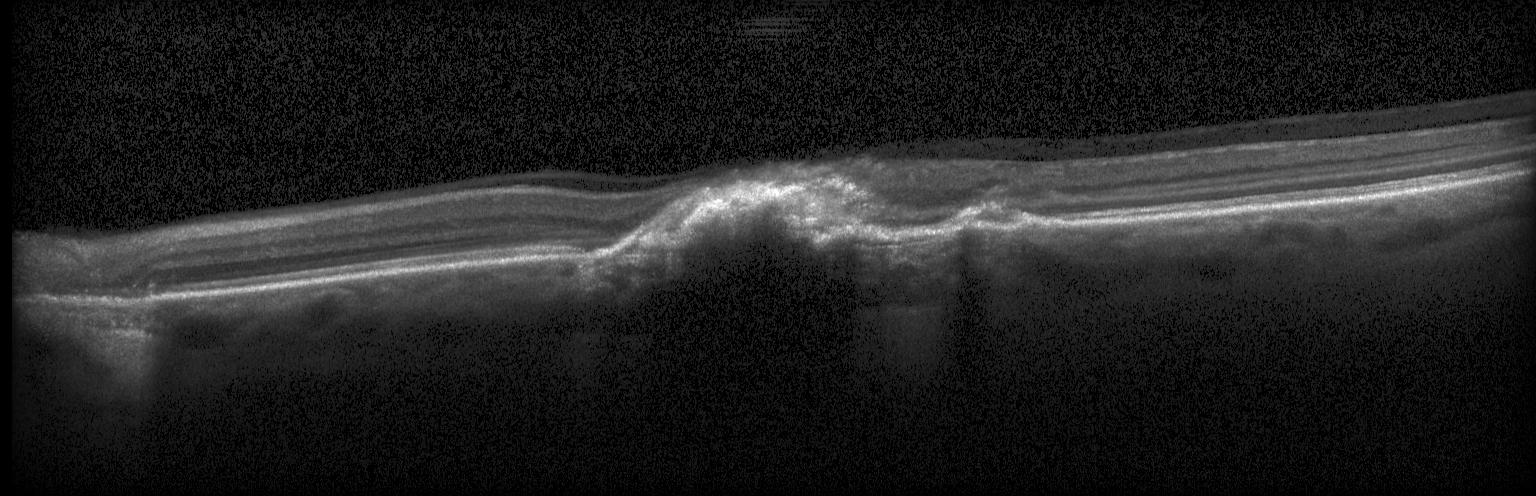 Retinal OCT cross-section. Impression: a choroidal neovascular membrane.